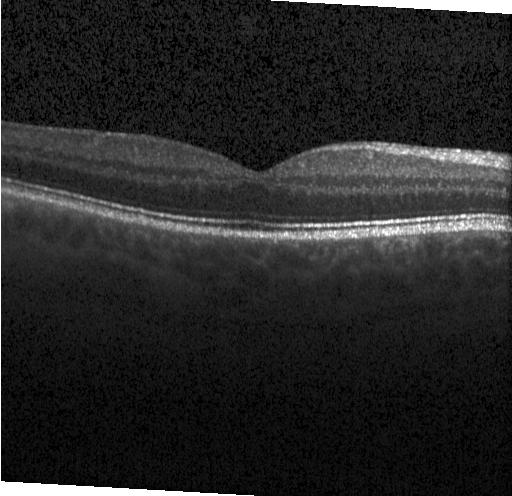 The scan shows neither CNV, DME, nor drusen.